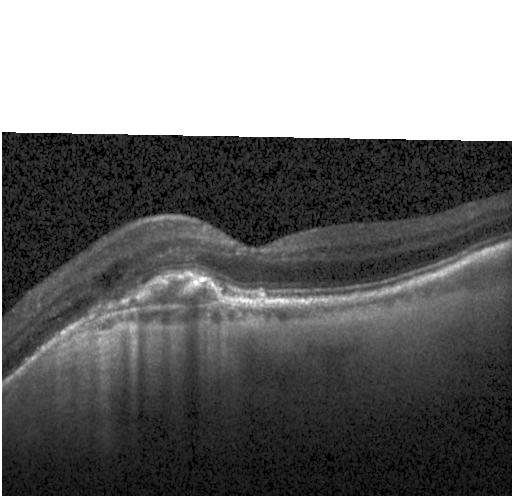 Macular OCT: a choroidal neovascular membrane.